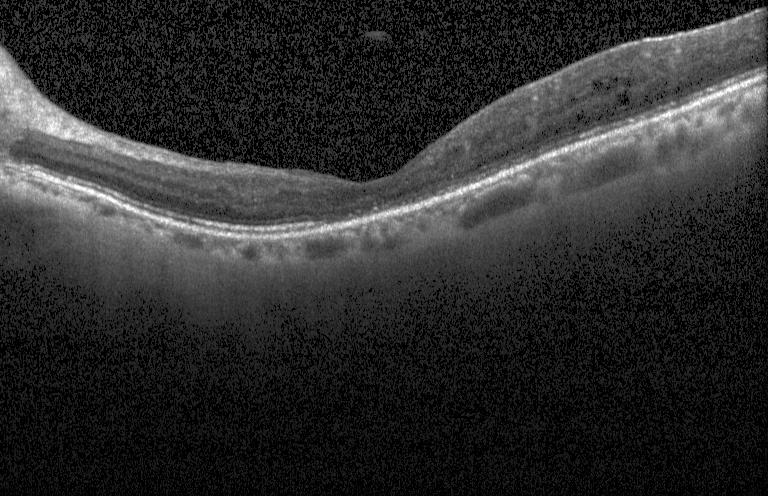 OCT B-scan; instrument: Heidelberg Spectralis — Diabetic macular edema.